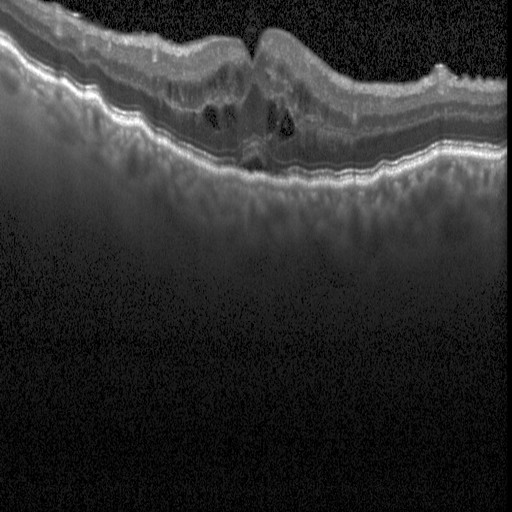

Optical coherence tomography B-scan · SD-OCT · Heidelberg Spectralis OCT system.
Finding: diabetic macular edema.